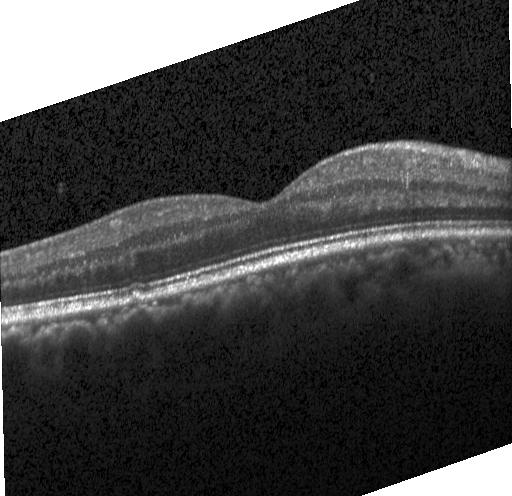

Finding: multiple drusen.